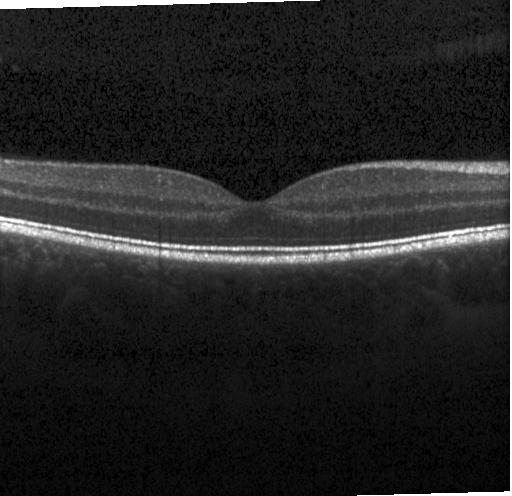
Retinal OCT cross-section · Heidelberg Spectralis · SD-OCT
Diagnosis: neither CNV, DME, nor drusen.